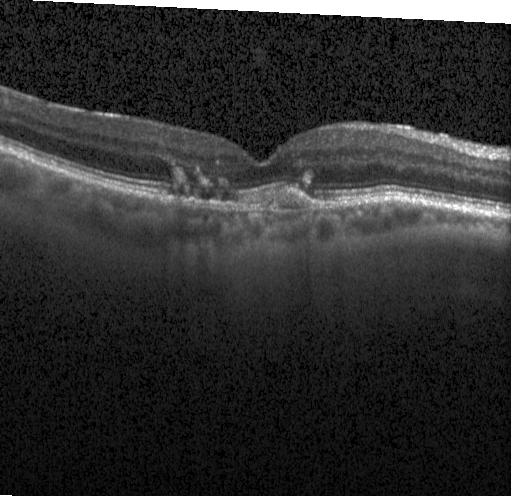 Instrument: Heidelberg Spectralis. Horizontal scan through the fovea. Retinal OCT B-scan.
Finding: choroidal neovascularization (CNV).